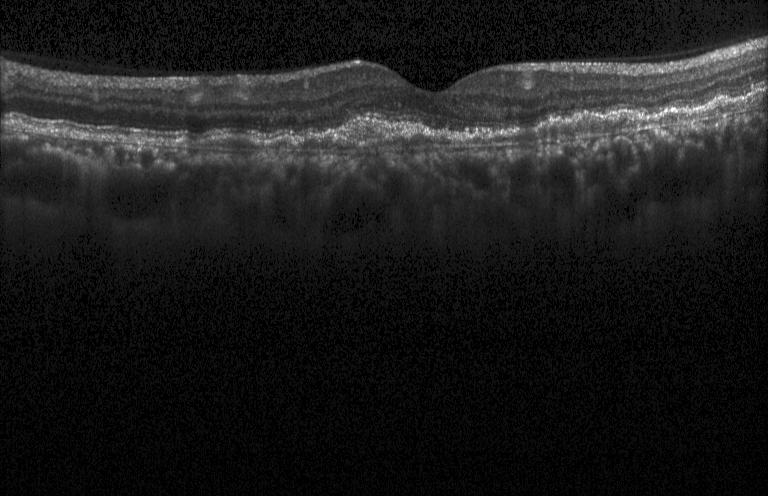

Centered on the fovea, optical coherence tomography scan
OCT finding: a choroidal neovascular membrane.